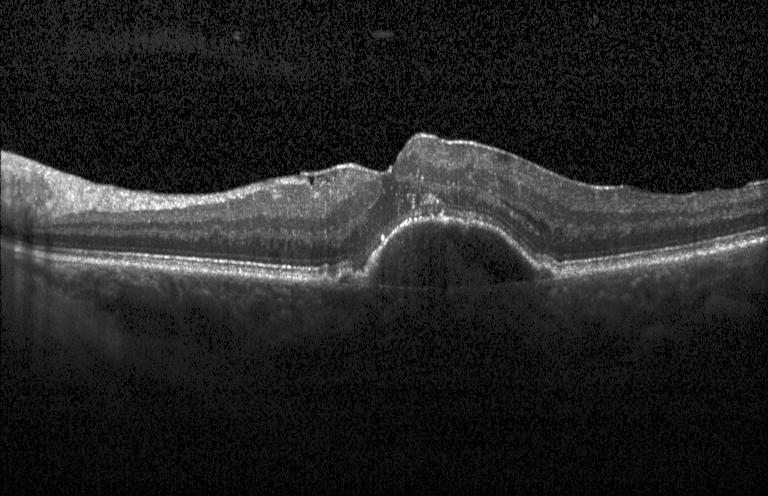

Optical coherence tomography scan, spectral-domain OCT, macular scan
Assessment: a choroidal neovascular membrane.